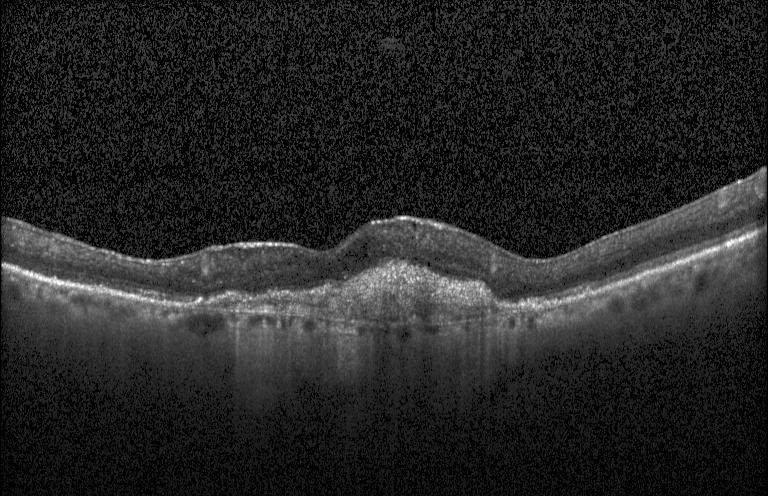 Optical coherence tomography scan, spectral-domain OCT. Assessment: a choroidal neovascular membrane.